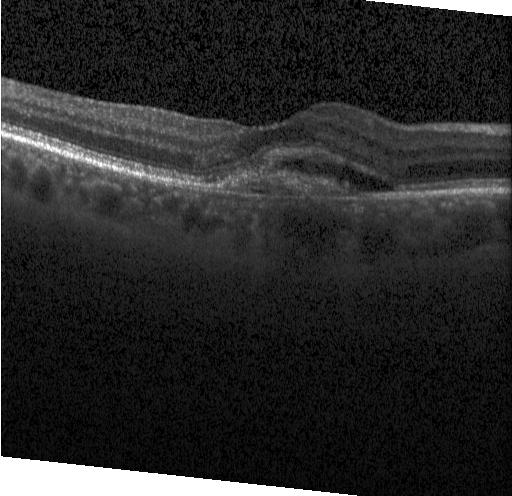
OCT scan showing CNV.